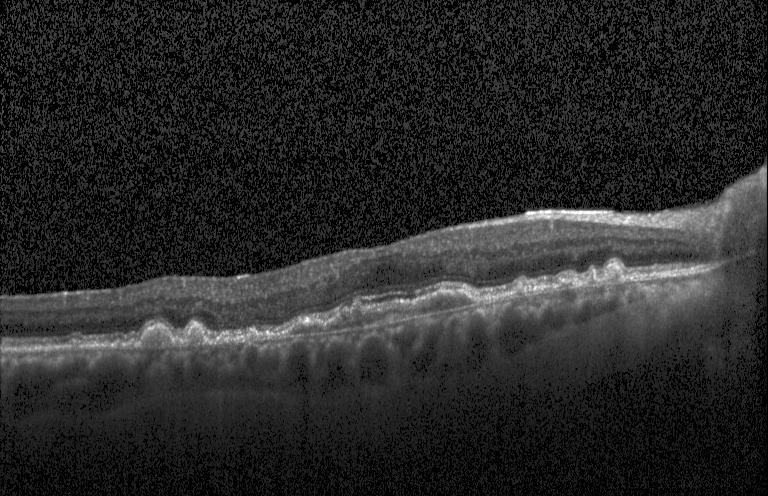 Centered on the fovea. Spectral-domain optical coherence tomography. OCT line scan. Heidelberg Spectralis OCT system. Diagnosis: choroidal neovascularization.